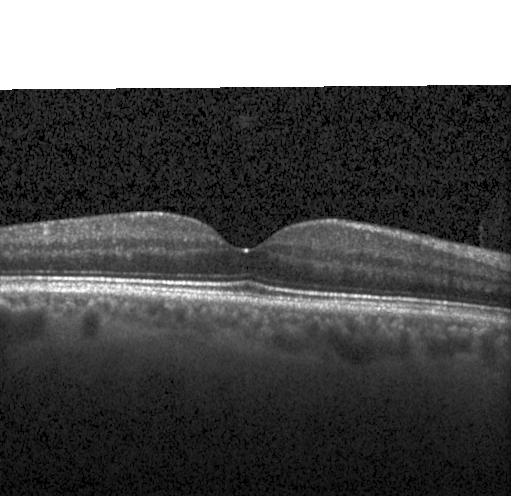
OCT finding: no choroidal neovascularization, diabetic macular edema, or drusen.